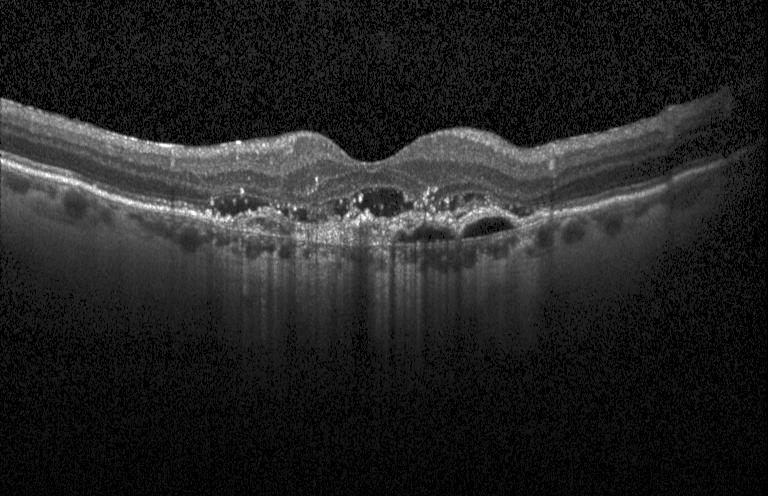

Dx: a choroidal neovascular membrane.